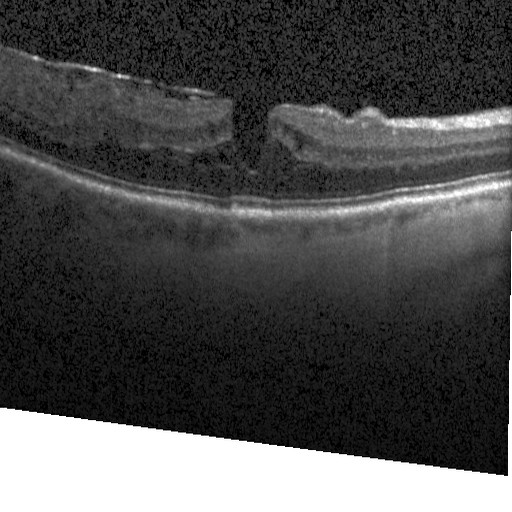
Acquired on a Heidelberg Spectralis. Optical coherence tomography scan. Macular scan
Impression: DME.